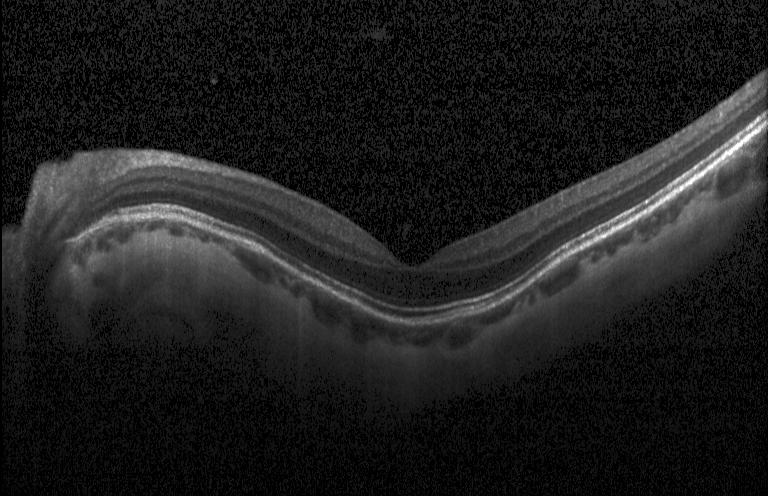 Spectral-domain optical coherence tomography; OCT B-scan. Finding: no evidence of choroidal neovascularization, diabetic macular edema, or drusen.